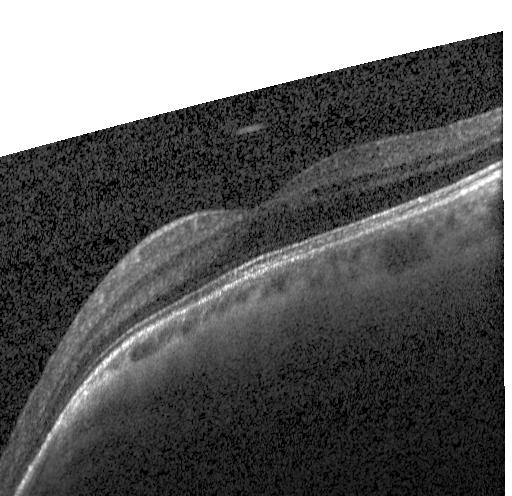

Spectral-domain OCT B-scan: no evidence of choroidal neovascularization, diabetic macular edema, or drusen.